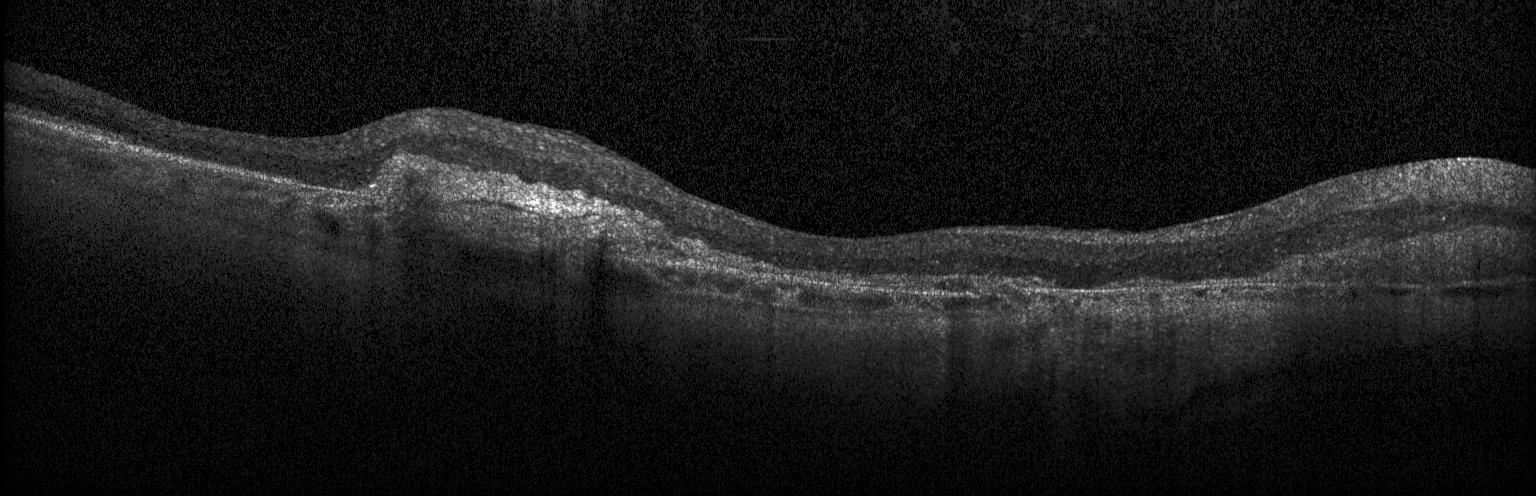
OCT line scan
Impression: CNV.